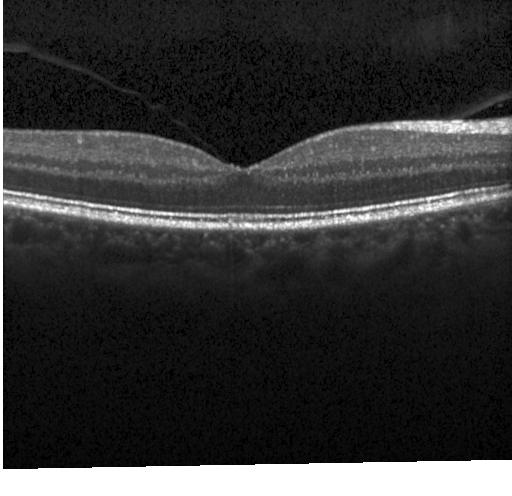

Macular OCT demonstrating no choroidal neovascularization, diabetic macular edema, or drusen.